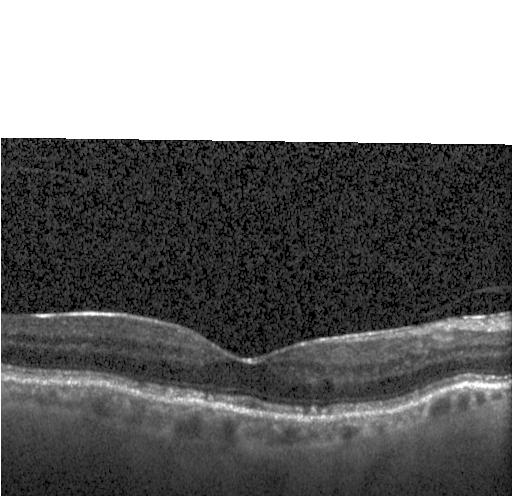 Diagnosis: neither choroidal neovascularization, diabetic macular edema, nor drusen.